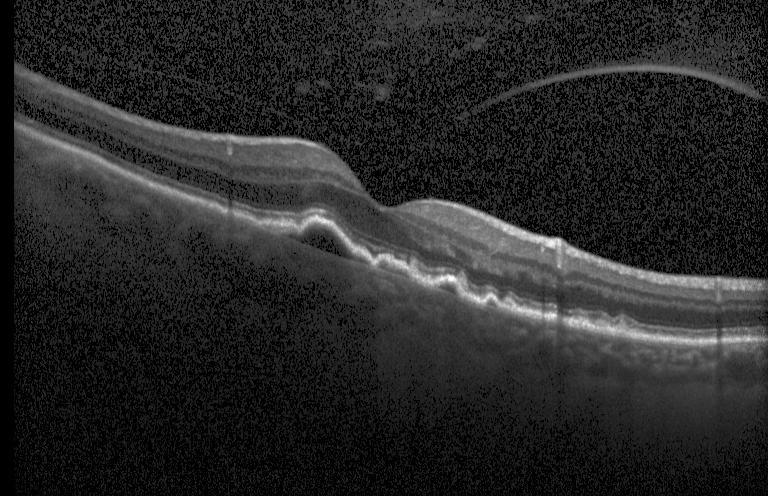

Spectral-domain OCT B-scan: a choroidal neovascular membrane.